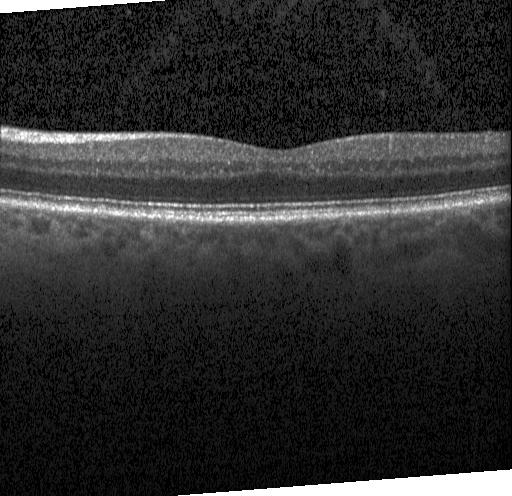

OCT scan showing no choroidal neovascularization, diabetic macular edema, or drusen.